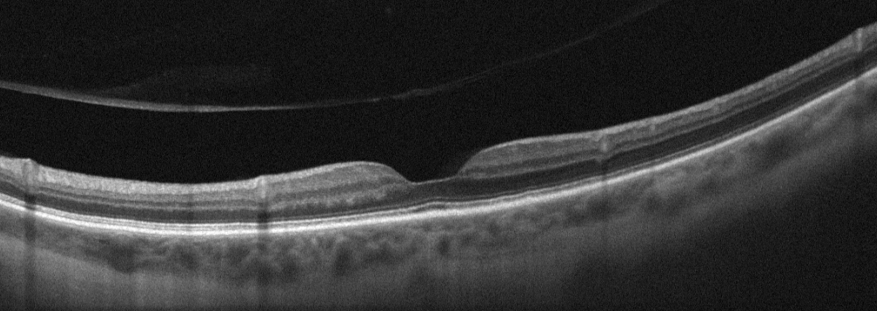
Optical coherence tomography scan. Macular OCT: absence of AMD, DME, ERM, RAO, RVO, and vitreomacular interface disease.